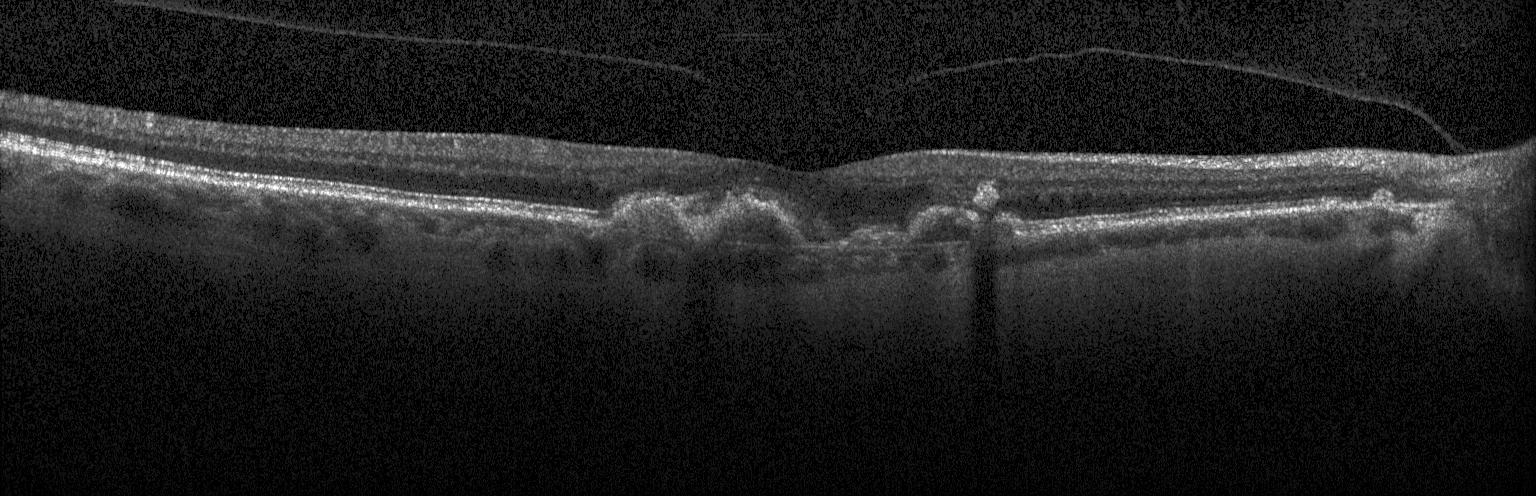 Macular OCT: choroidal neovascularization (CNV).